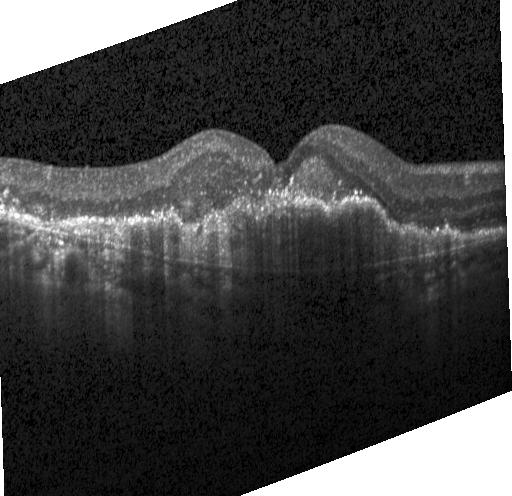 Retinal OCT cross-section; spectral-domain OCT — The scan shows choroidal neovascularization (CNV).